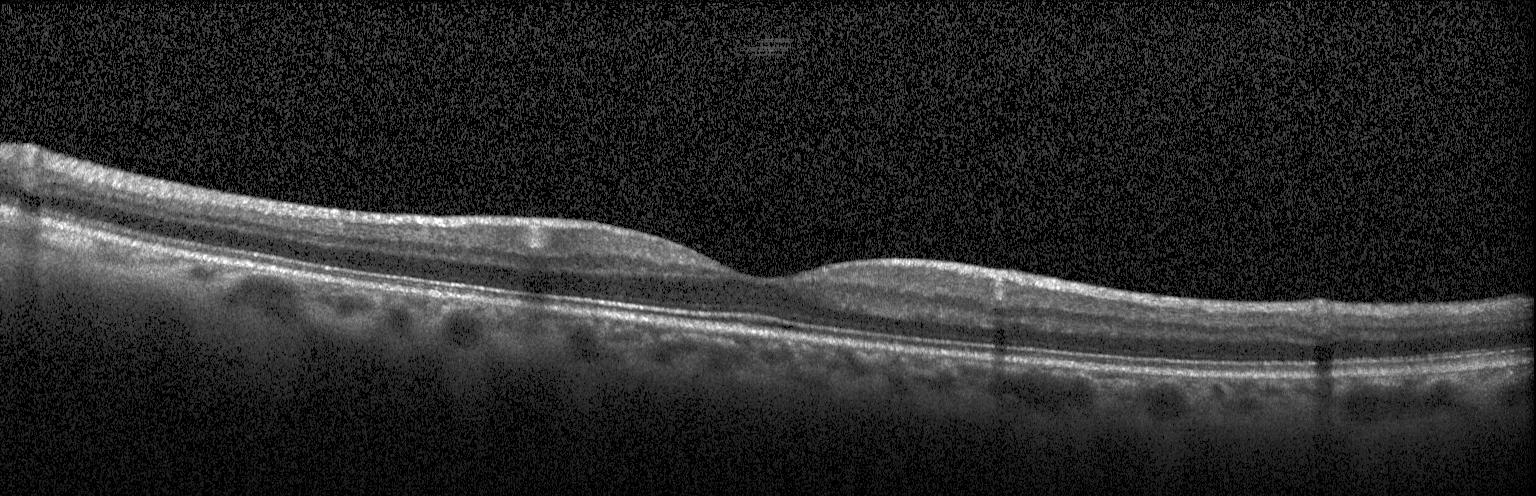

OCT B-scan
Finding: no evidence of CNV, DME, or drusen.